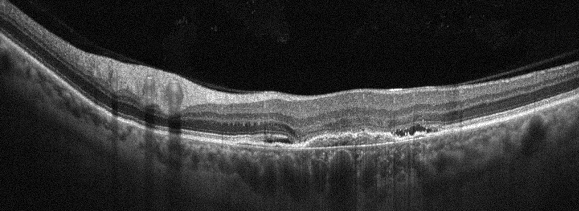 Optical coherence tomography B-scan. OS — Finding: AMD.